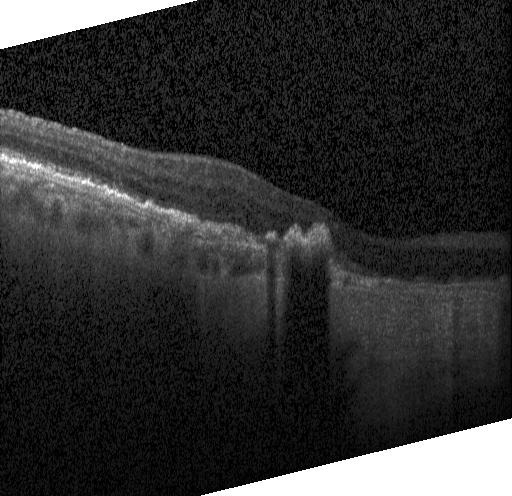 Diagnosis: a choroidal neovascular membrane.